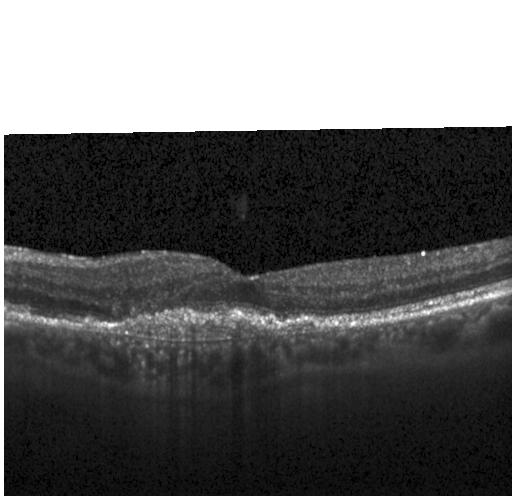

Diagnosis: a choroidal neovascular membrane.